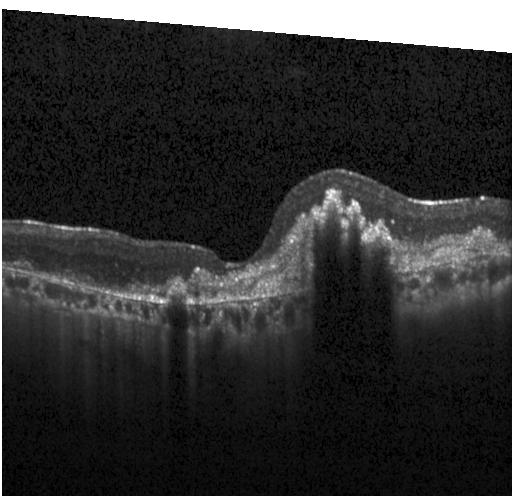 Assessment: a choroidal neovascular membrane.